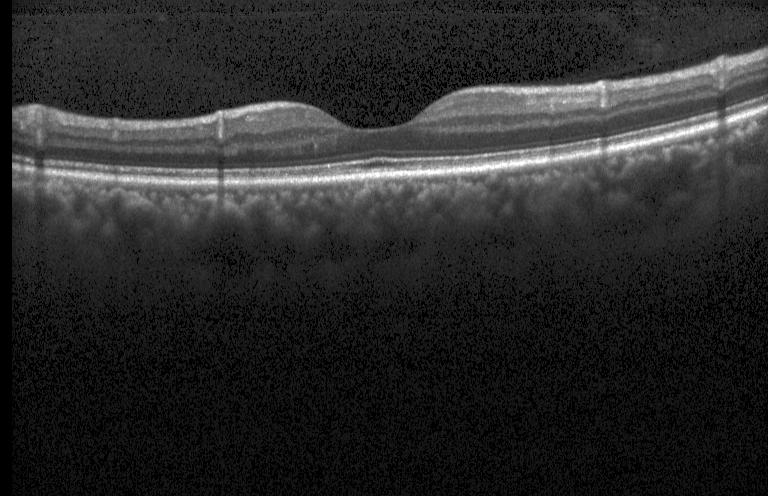 Dx: neither choroidal neovascularization, diabetic macular edema, nor drusen.